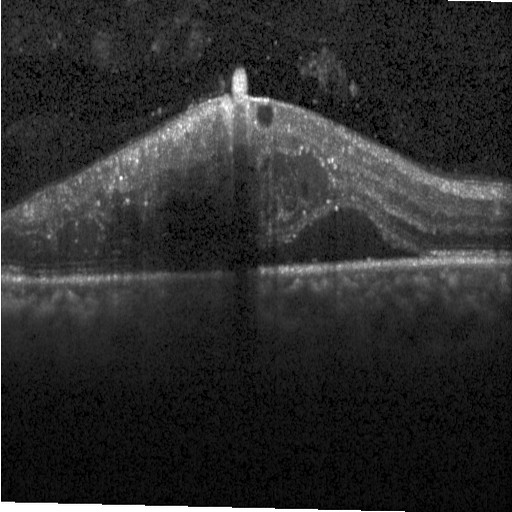
The scan shows DME.